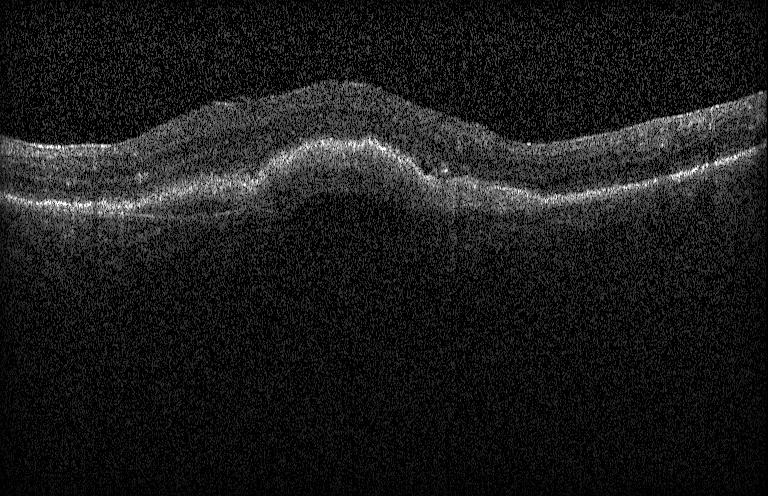

This B-scan demonstrates a choroidal neovascular membrane.